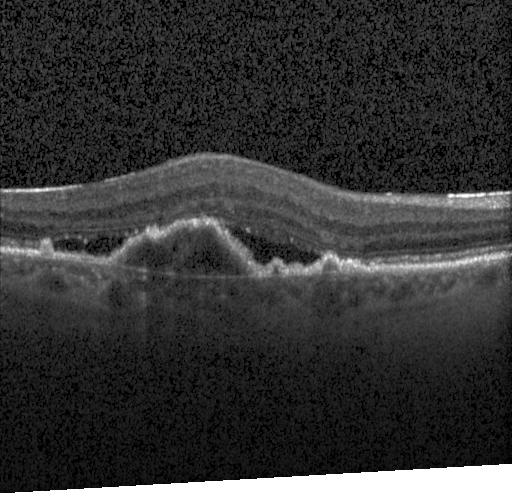 Centered on the fovea, spectral-domain OCT, OCT line scan
The scan shows choroidal neovascularization (CNV).